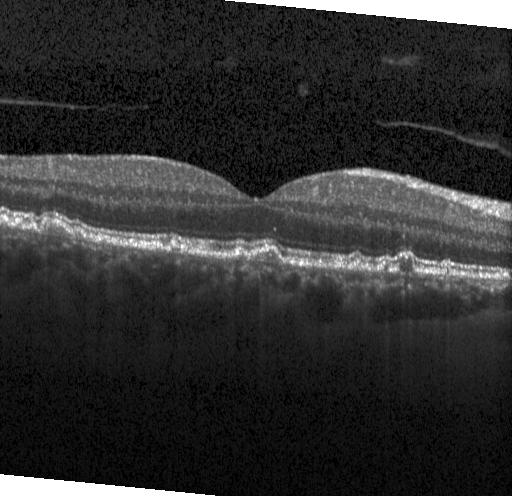
Macular scan; Heidelberg Spectralis OCT system; retinal OCT cross-section
Impression: sub-RPE drusenoid deposits.